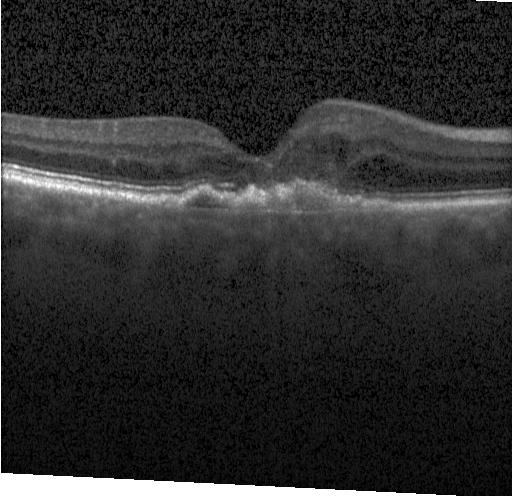 Diagnosis: a choroidal neovascular membrane.